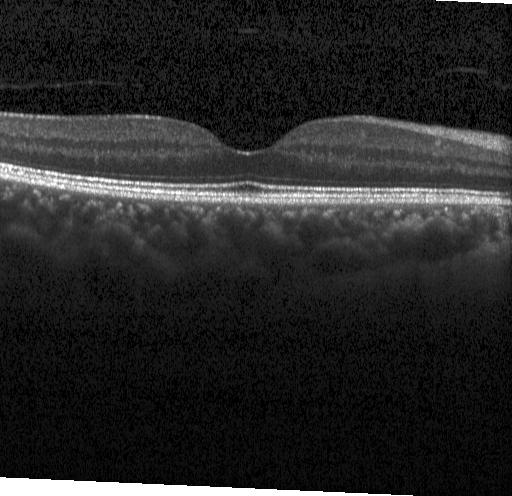 Neither CNV, DME, nor drusen.